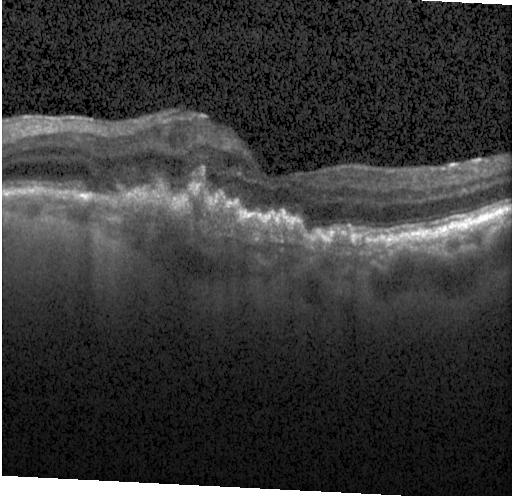
Retinal OCT cross-section, Heidelberg Spectralis OCT system. Dx: a choroidal neovascular membrane.